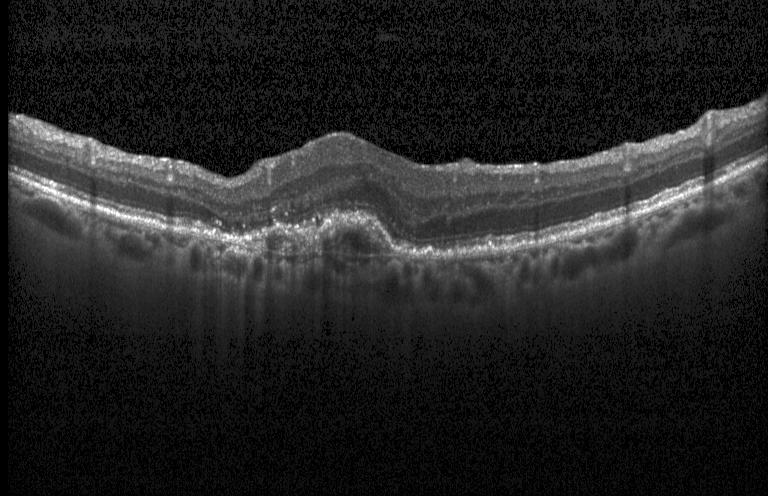
Finding: choroidal neovascularization (CNV).